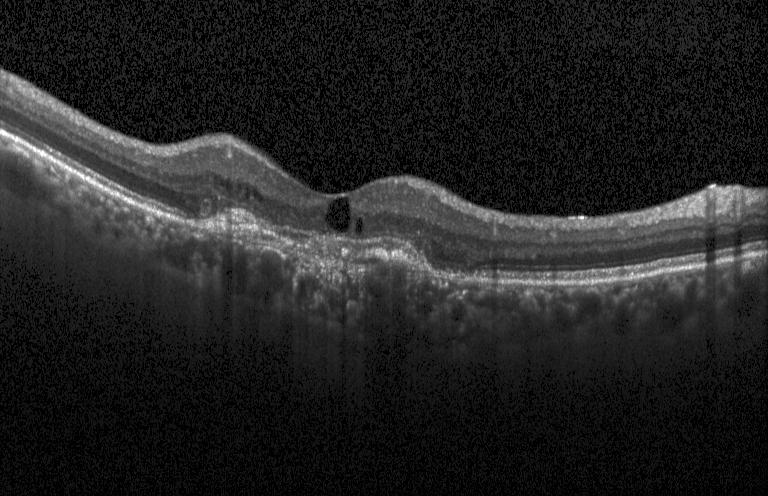 Spectral-domain OCT. Heidelberg Spectralis. OCT line scan. Horizontal scan through the fovea — The scan shows CNV.